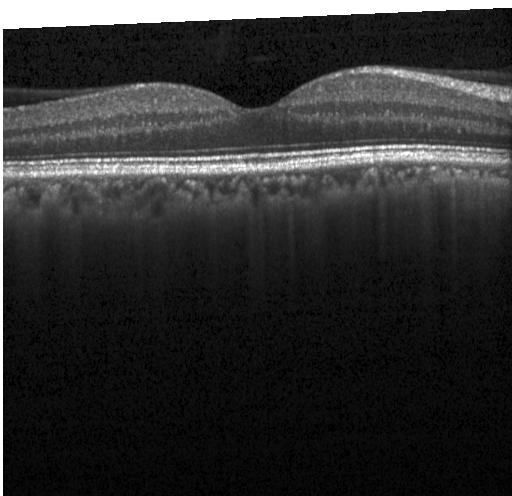

This B-scan demonstrates no CNV, no DME, and no drusen.